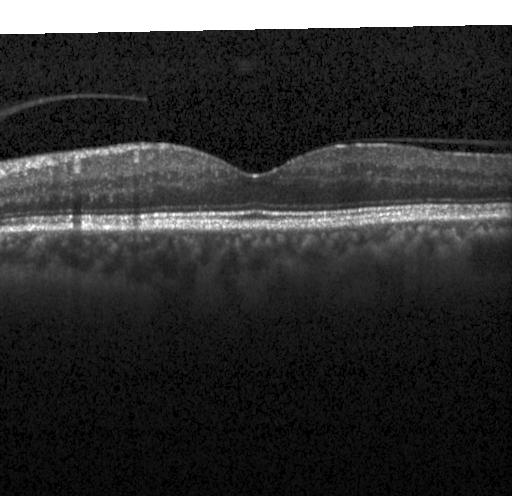 Optical coherence tomography scan, spectral-domain OCT. Impression: no evidence of CNV, DME, or drusen.